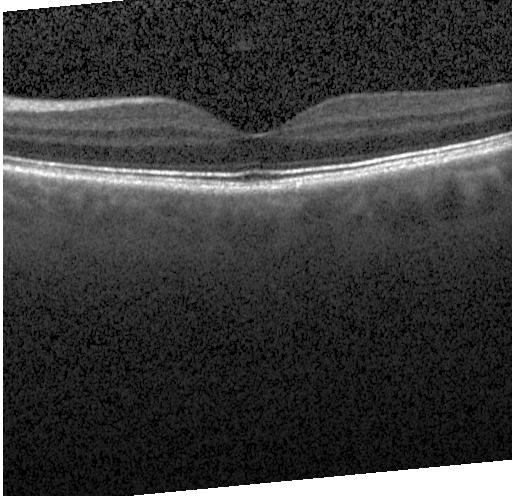
Centered on the fovea · retinal OCT cross-section · instrument: Heidelberg Spectralis — OCT finding: no choroidal neovascularization, no diabetic macular edema, and no drusen.